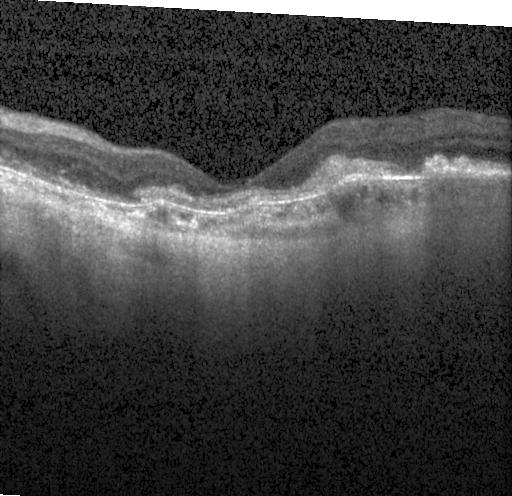 OCT B-scan showing CNV.